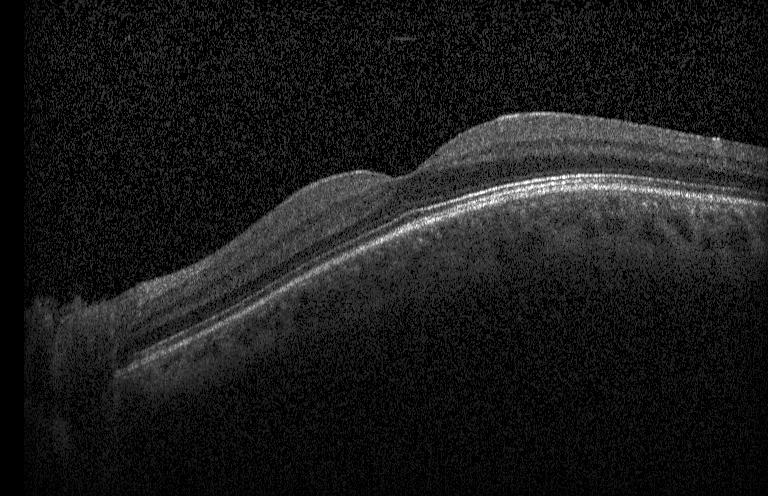

Optical coherence tomography scan
Assessment: no choroidal neovascularization, diabetic macular edema, or drusen.